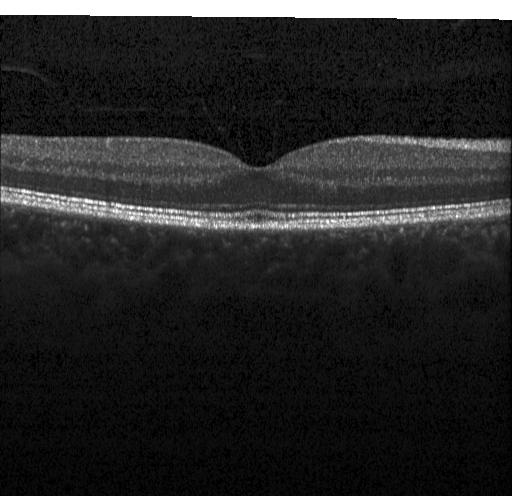

Horizontal scan through the fovea. SD-OCT. Optical coherence tomography scan — Finding: no choroidal neovascularization, no diabetic macular edema, and no drusen.